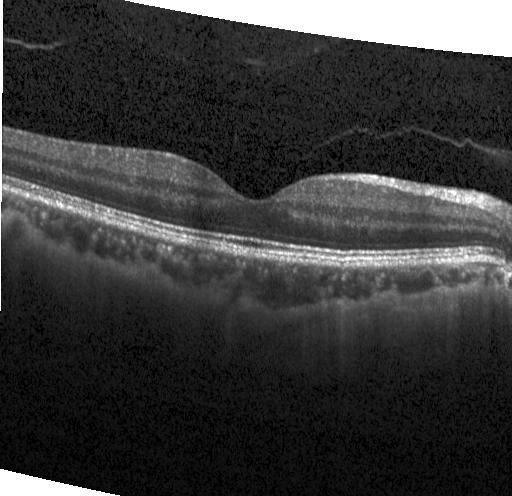 Spectral-domain OCT, retinal OCT B-scan, horizontal scan through the fovea, Heidelberg Spectralis OCT system
Diagnosis: no choroidal neovascularization, diabetic macular edema, or drusen.